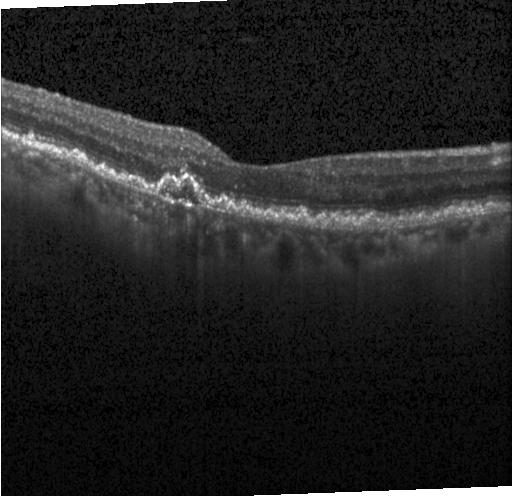 Dx: a choroidal neovascular membrane.